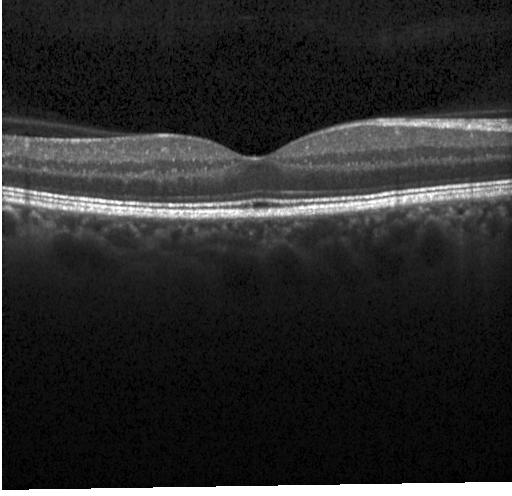
Retinal OCT cross-section · centered on the fovea.
Assessment: no CNV, DME, or drusen.